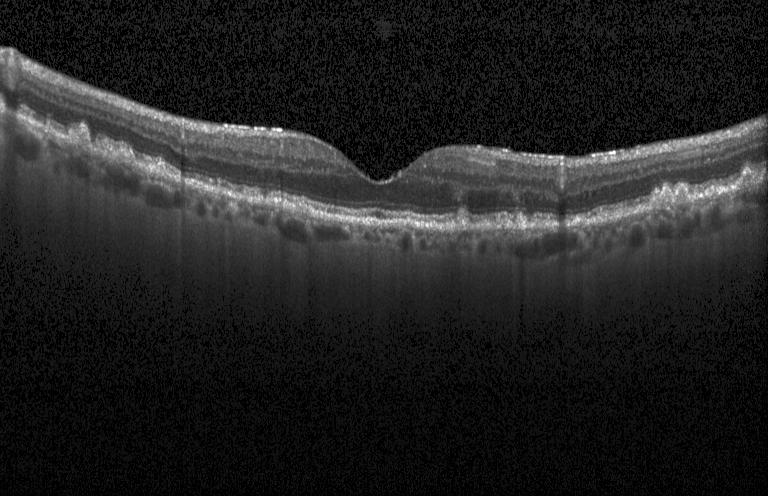

OCT line scan. Impression: sub-RPE drusenoid deposits.